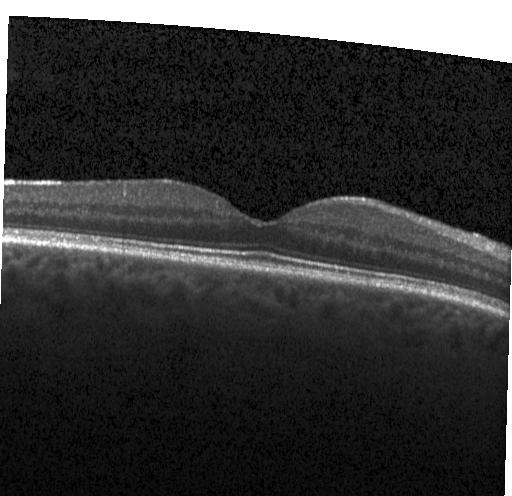

OCT scan showing no evidence of choroidal neovascularization, diabetic macular edema, or drusen.